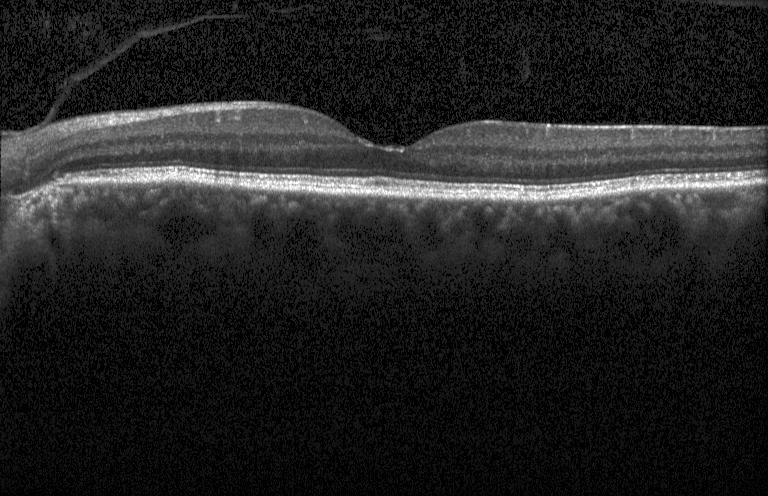

OCT line scan — Diagnosis: neither choroidal neovascularization, diabetic macular edema, nor drusen.